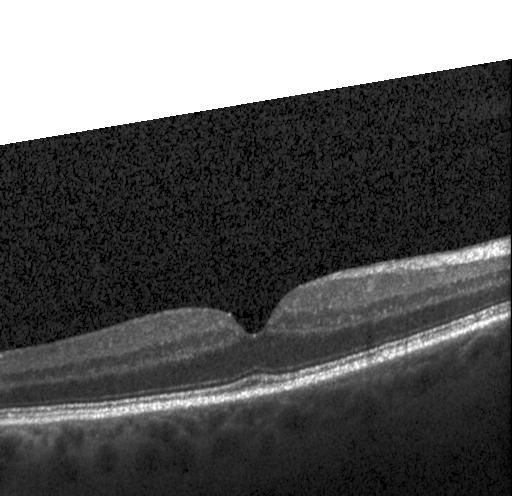
Spectral-domain OCT B-scan: neither choroidal neovascularization, diabetic macular edema, nor drusen.